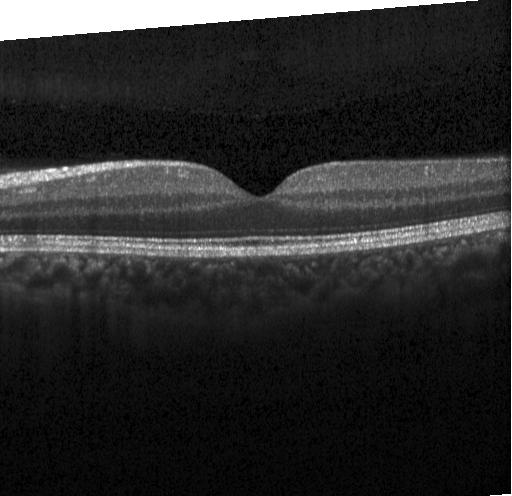

Macular scan, instrument: Heidelberg Spectralis, OCT B-scan, spectral-domain OCT
OCT finding: neither choroidal neovascularization, diabetic macular edema, nor drusen.